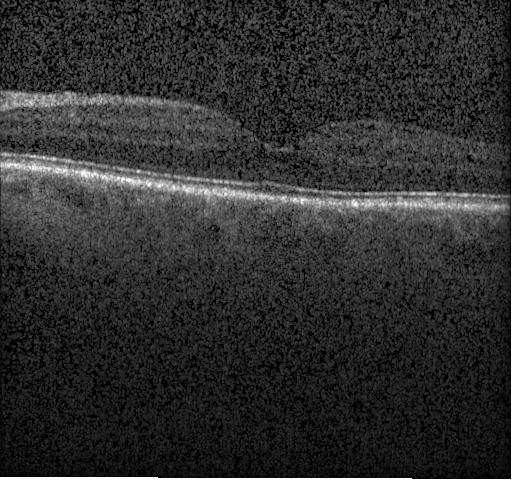
OCT scan showing no choroidal neovascularization, diabetic macular edema, or drusen.